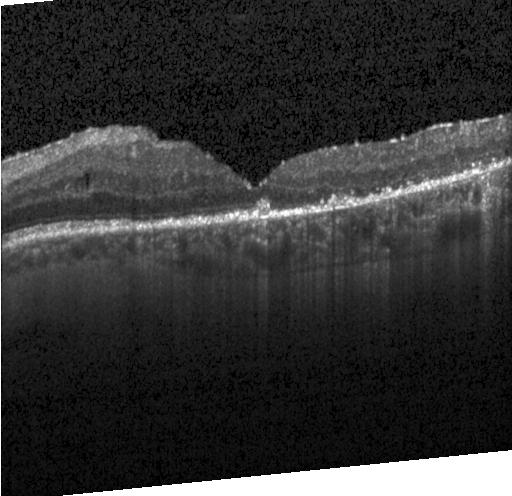

The scan shows diabetic macular edema (DME).